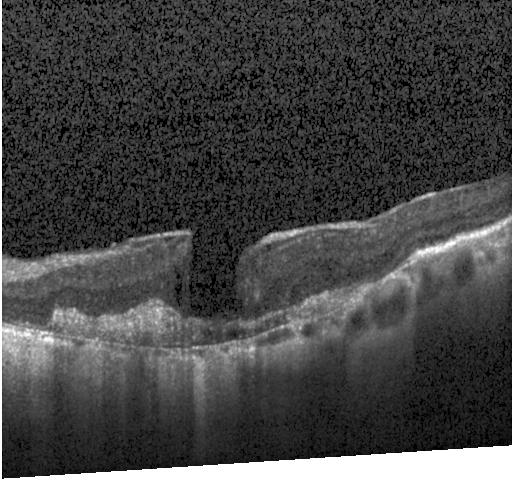 Spectral-domain OCT B-scan: CNV.